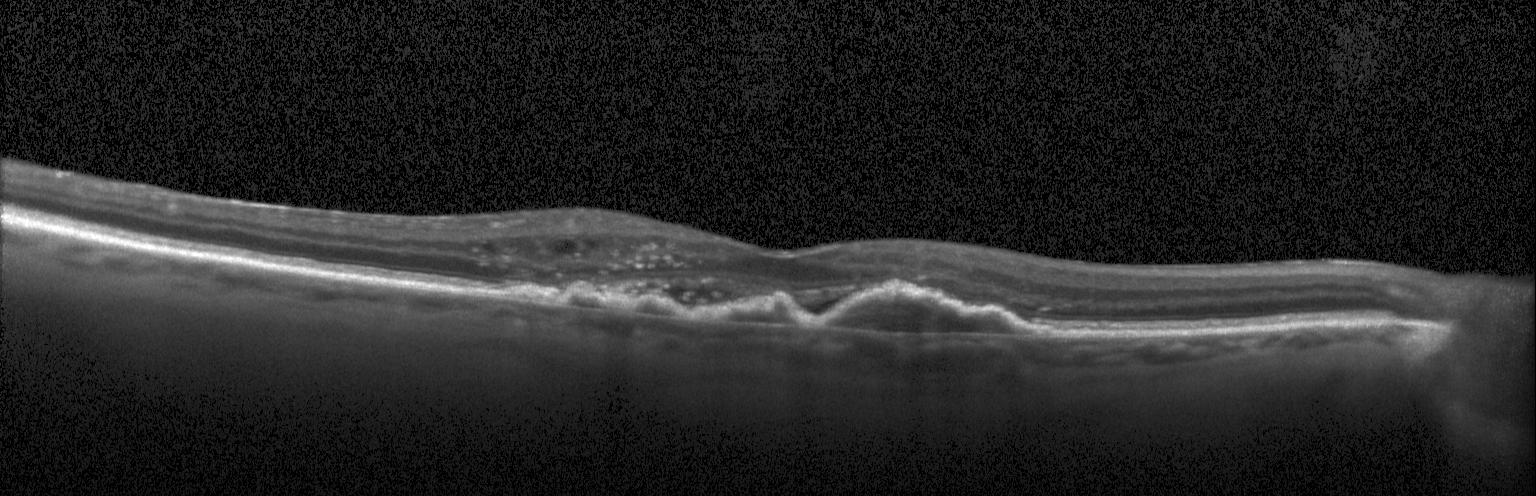
Spectral-domain OCT; optical coherence tomography scan; Heidelberg Spectralis
Impression: a choroidal neovascular membrane.